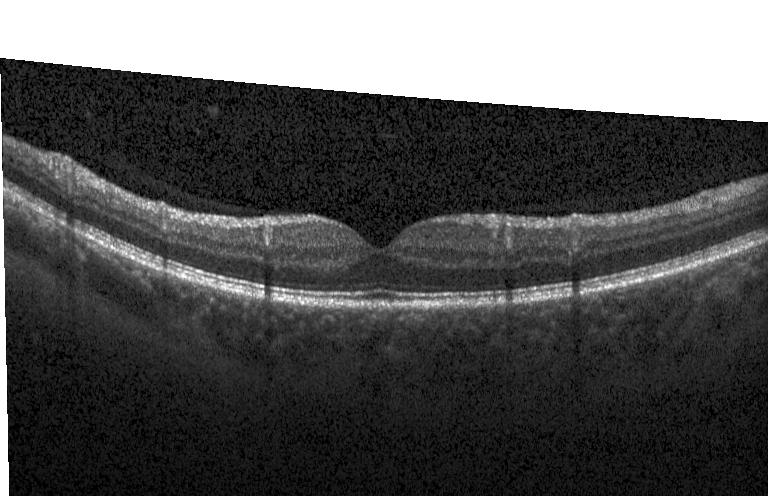

This B-scan demonstrates no evidence of choroidal neovascularization, diabetic macular edema, or drusen.